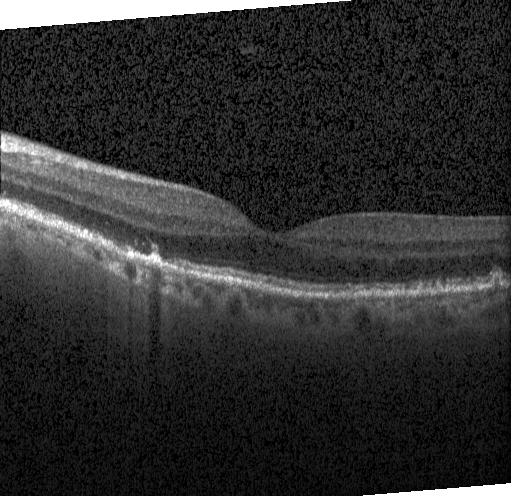
Macular OCT: drusen.